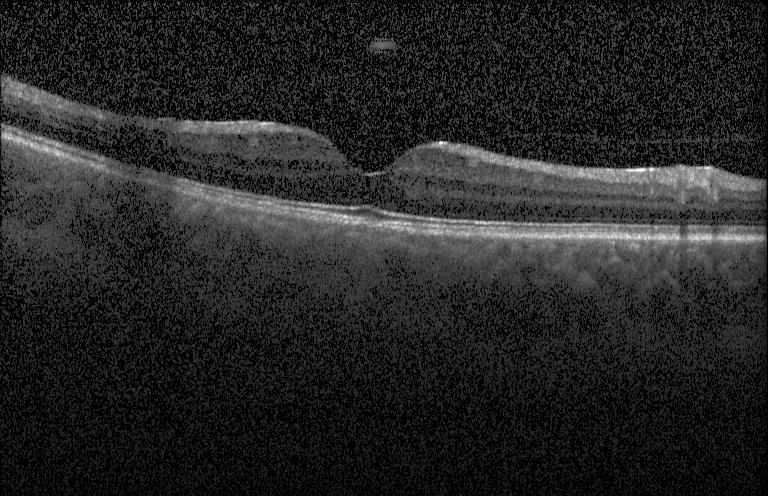
OCT B-scan
Impression: no CNV, no DME, and no drusen.